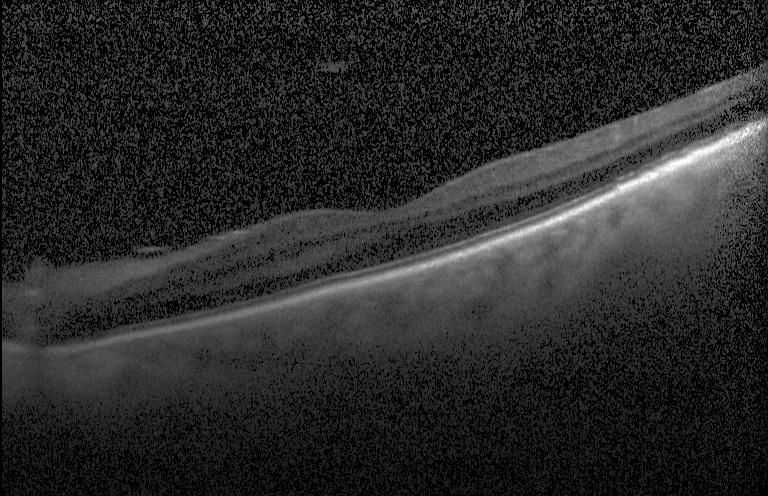 Diagnosis: no choroidal neovascularization, no diabetic macular edema, and no drusen.